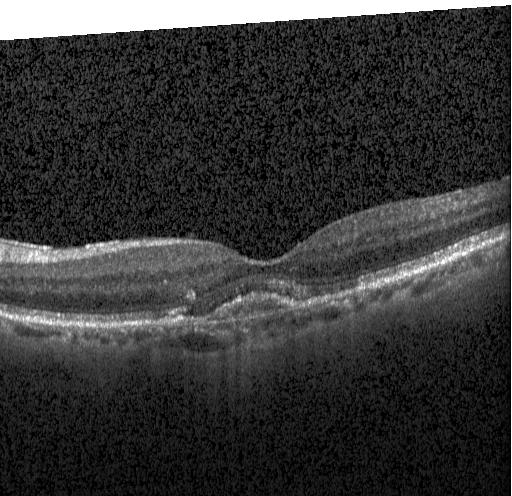
Optical coherence tomography B-scan; through the macula; Heidelberg Spectralis. Impression: choroidal neovascularization (CNV).